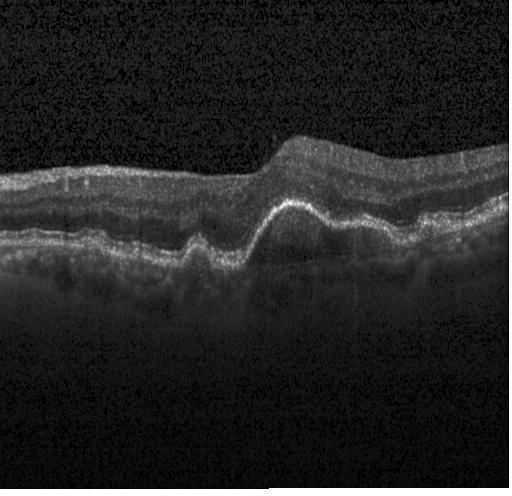 OCT scan showing sub-RPE drusenoid deposits.